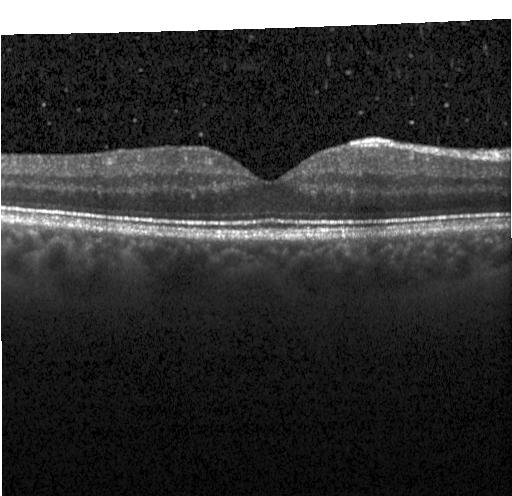 Acquired on a Heidelberg Spectralis · spectral-domain optical coherence tomography · retinal OCT B-scan. OCT finding: no choroidal neovascularization, diabetic macular edema, or drusen.